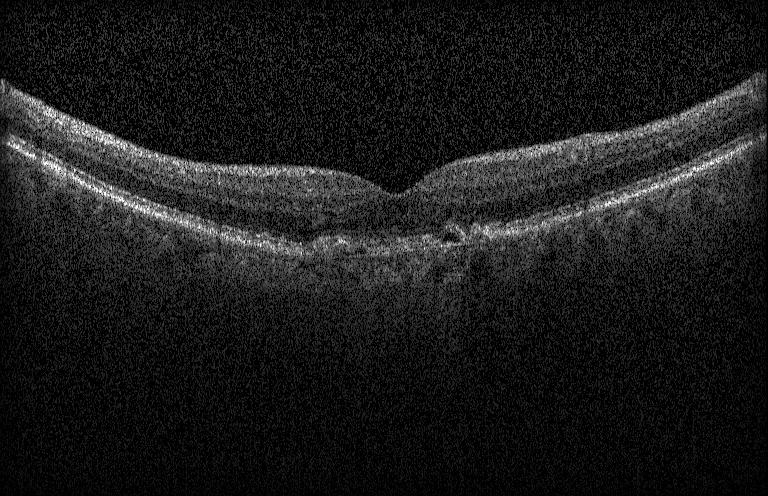 OCT finding: CNV.